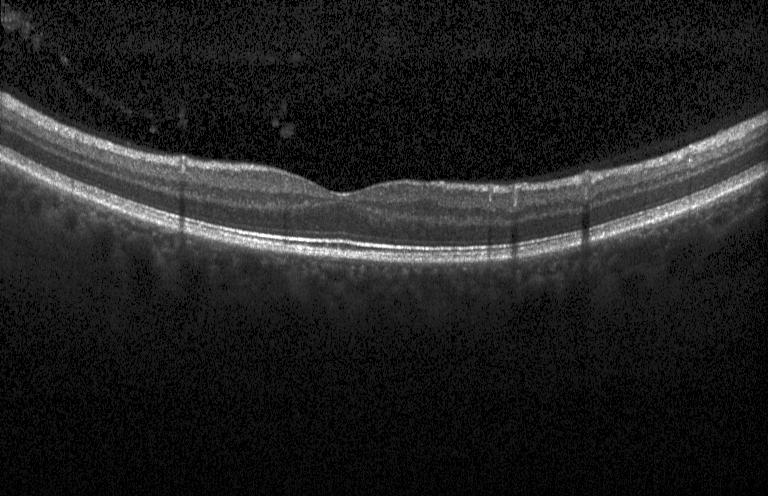
Spectral-domain OCT · retinal OCT B-scan · Heidelberg Spectralis OCT system
Finding: no choroidal neovascularization, no diabetic macular edema, and no drusen.